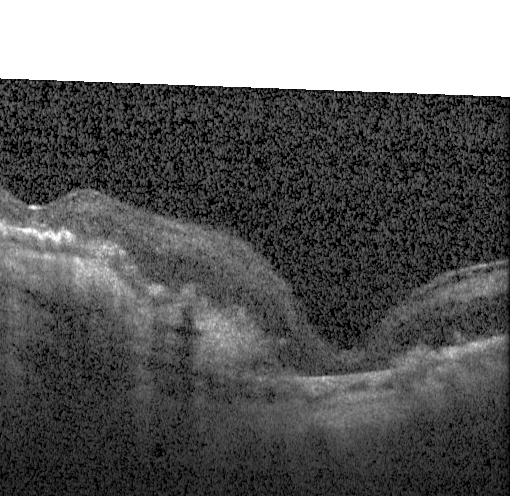 Finding: a choroidal neovascular membrane.